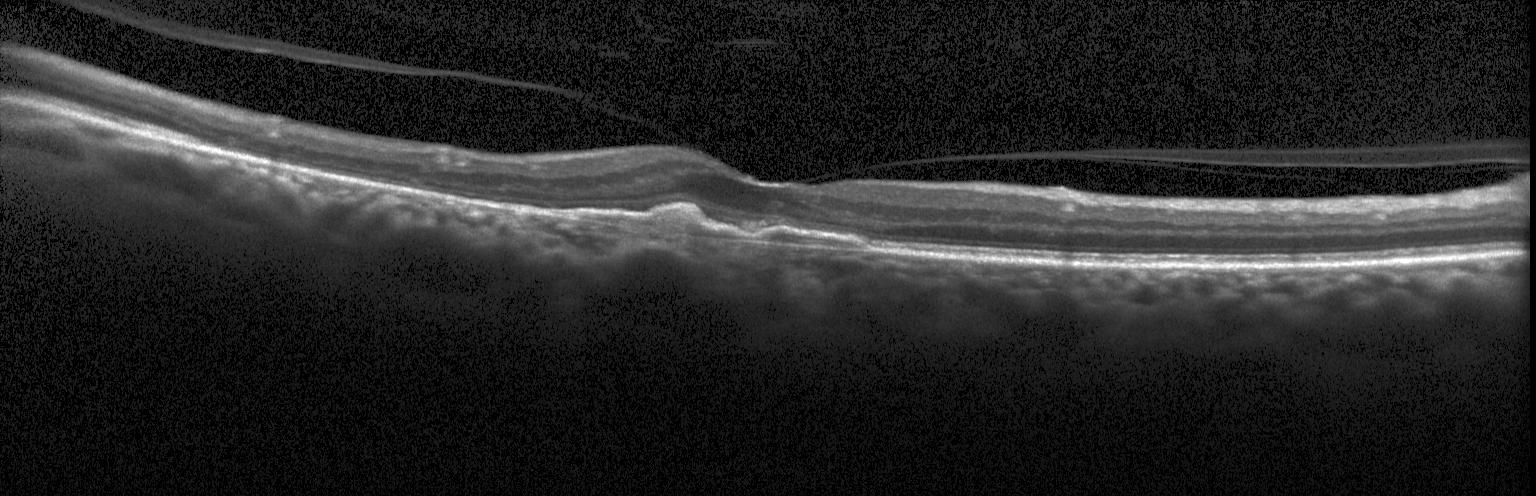 Heidelberg Spectralis, optical coherence tomography B-scan, fovea-centered — Assessment: a choroidal neovascular membrane.